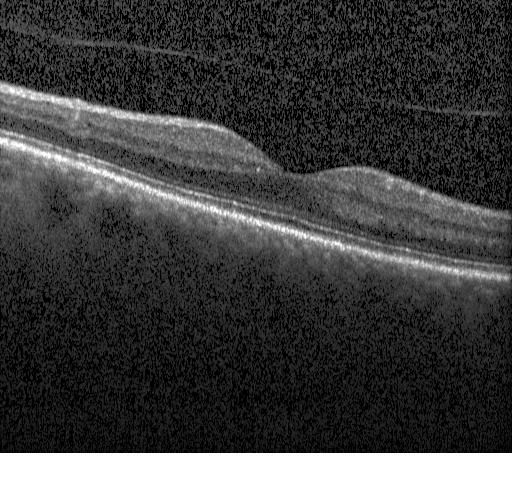 OCT B-scan · SD-OCT. The scan shows no CNV, DME, or drusen.